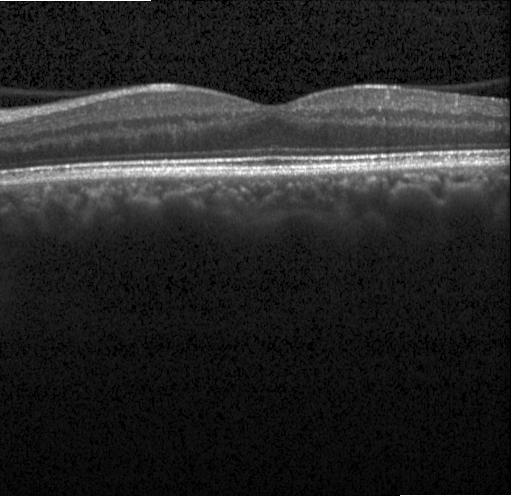

Acquired on a Heidelberg Spectralis, OCT line scan, spectral-domain OCT. The scan shows neither choroidal neovascularization, diabetic macular edema, nor drusen.